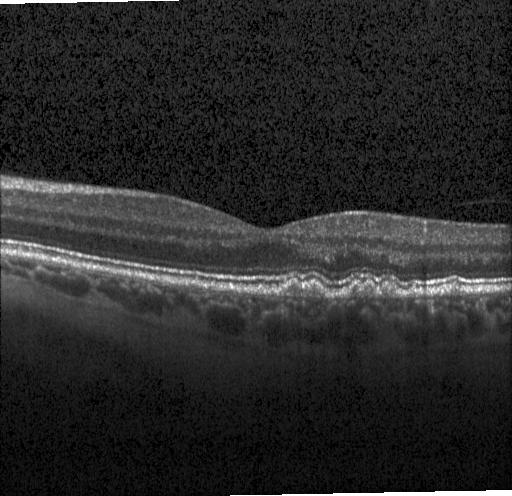 Diagnosis: drusen.